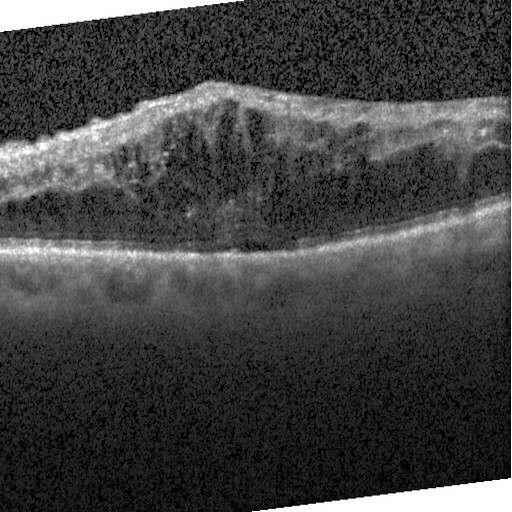
Retinal OCT cross-section showing diabetic macular edema (DME).